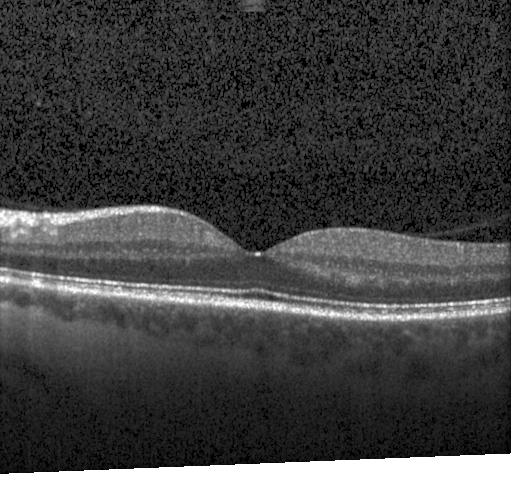 SD-OCT; OCT line scan — Finding: no choroidal neovascularization, no diabetic macular edema, and no drusen.